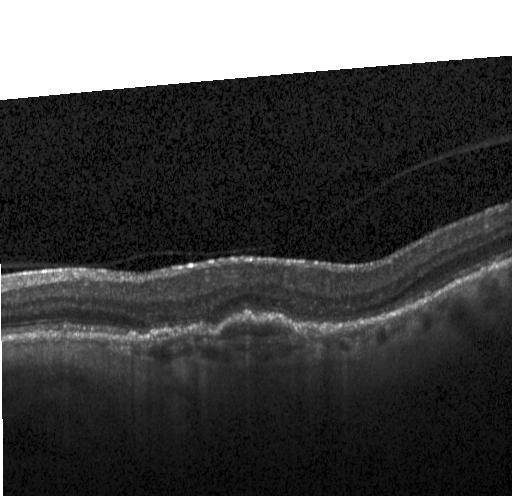 Finding: a choroidal neovascular membrane.